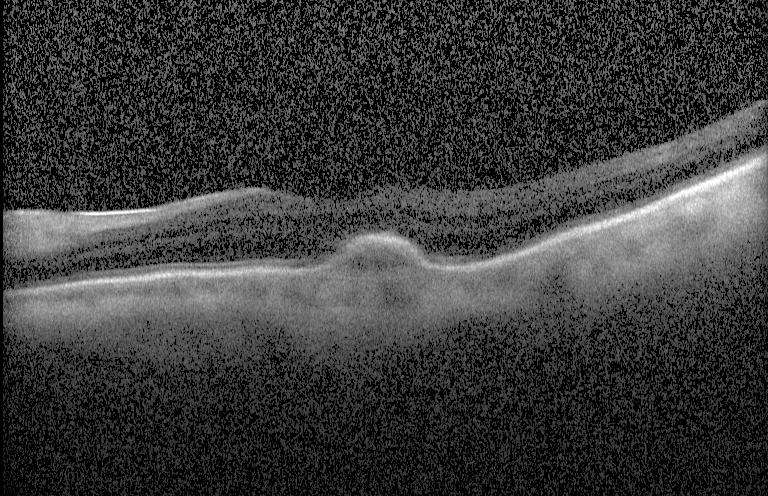 Optical coherence tomography scan, macular scan — Impression: choroidal neovascularization (CNV).